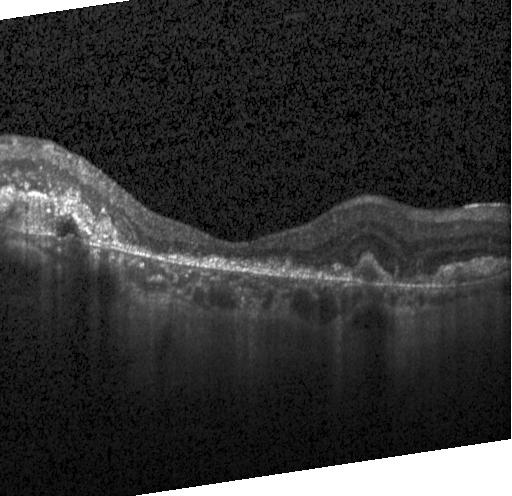
OCT B-scan · spectral-domain optical coherence tomography · Heidelberg Spectralis. Diagnosis: choroidal neovascularization.